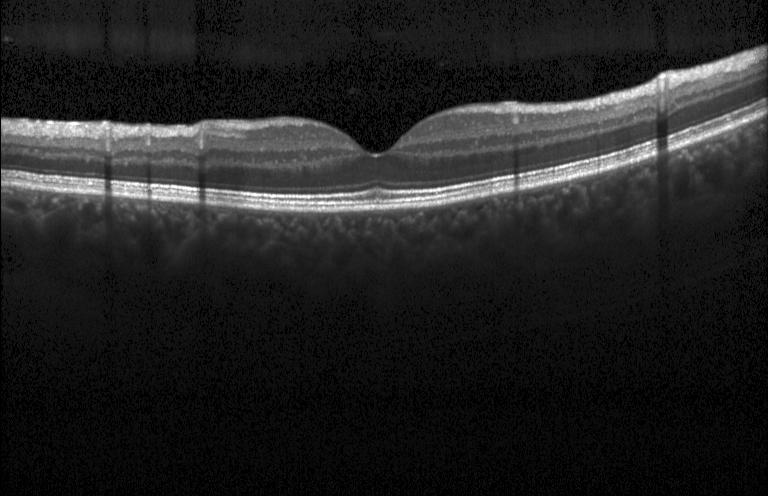
Macular OCT: neither choroidal neovascularization, diabetic macular edema, nor drusen.